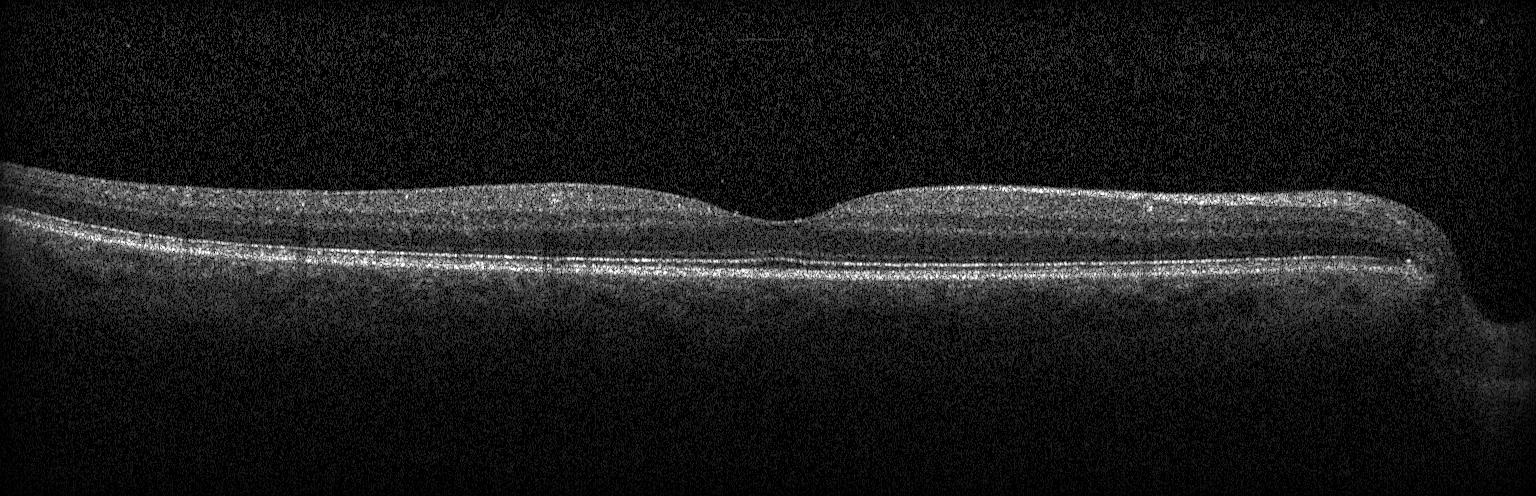

Dx: no evidence of CNV, DME, or drusen.